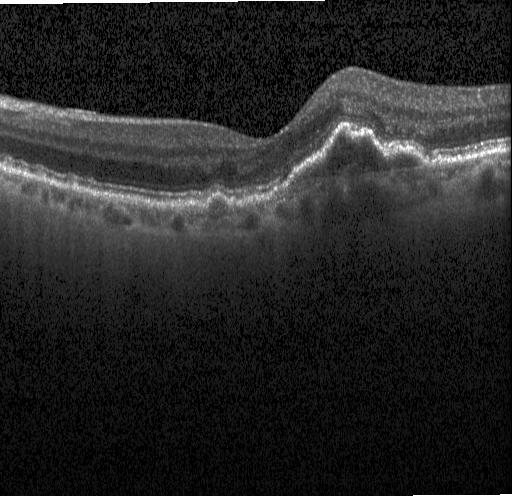
Optical coherence tomography scan
This B-scan demonstrates a choroidal neovascular membrane.